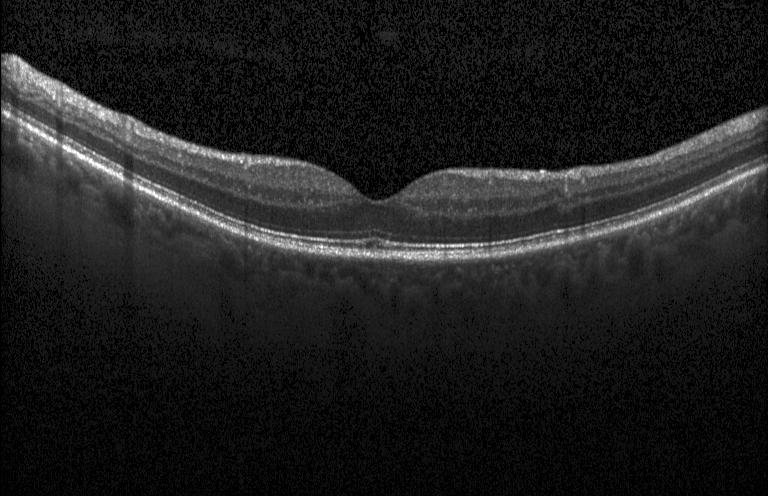
Optical coherence tomography B-scan, instrument: Heidelberg Spectralis.
Dx: no choroidal neovascularization, no diabetic macular edema, and no drusen.